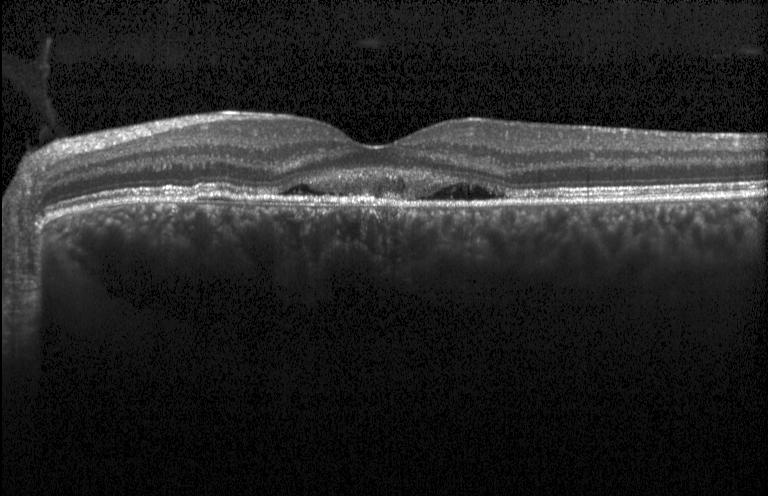

Instrument: Heidelberg Spectralis; horizontal scan through the fovea; spectral-domain OCT; retinal OCT B-scan.
Diagnosis: a choroidal neovascular membrane.